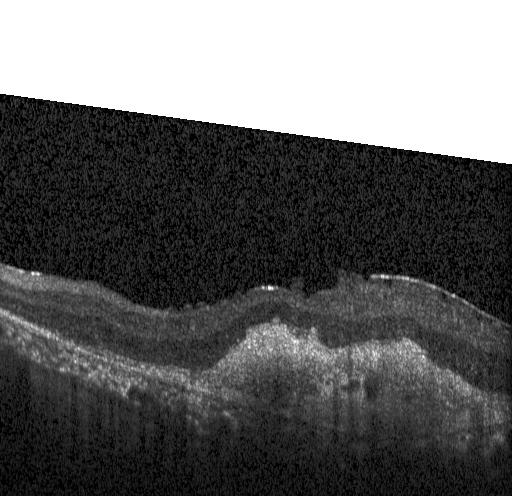 Horizontal scan through the fovea. Optical coherence tomography B-scan — Diagnosis: choroidal neovascularization (CNV).